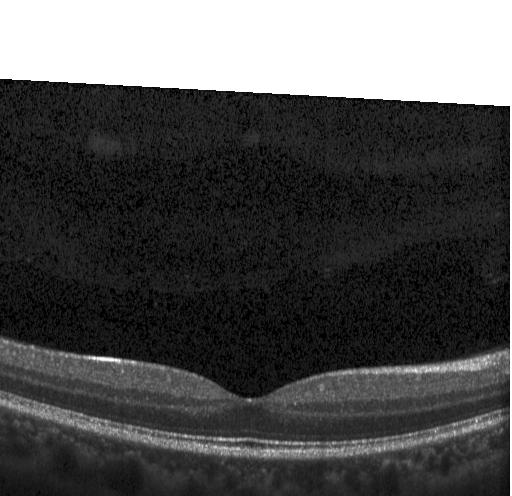
Dx: no CNV, no DME, and no drusen.